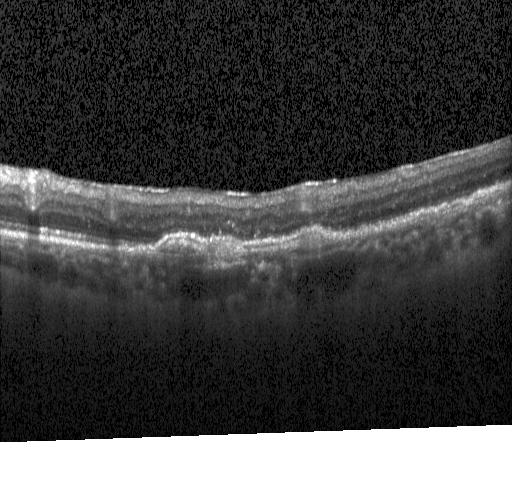

Retinal OCT cross-section
Diagnosis: a choroidal neovascular membrane.